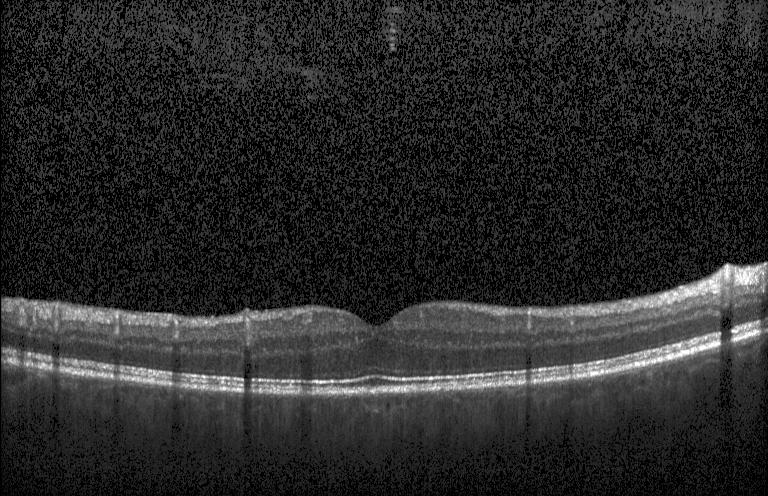 Retinal OCT cross-section
Diagnosis: no CNV, DME, or drusen.